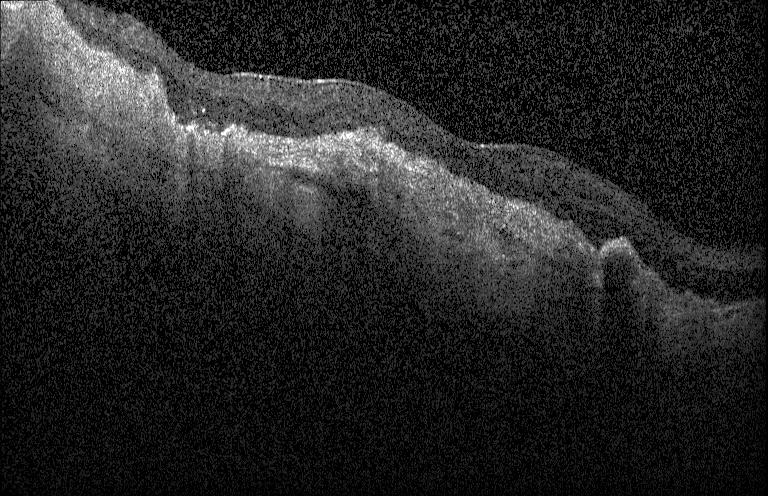

Optical coherence tomography B-scan — This B-scan demonstrates a choroidal neovascular membrane.